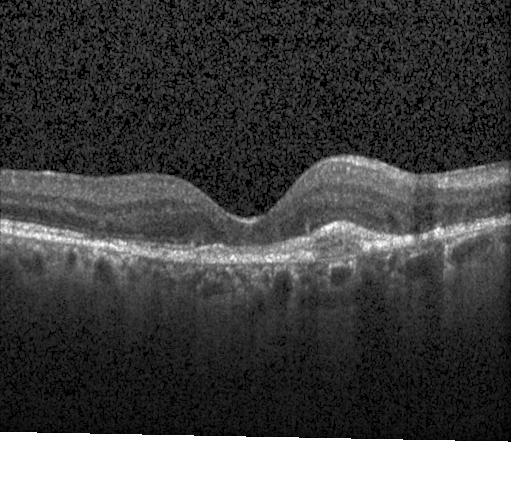 Retinal OCT cross-section — Impression: CNV.